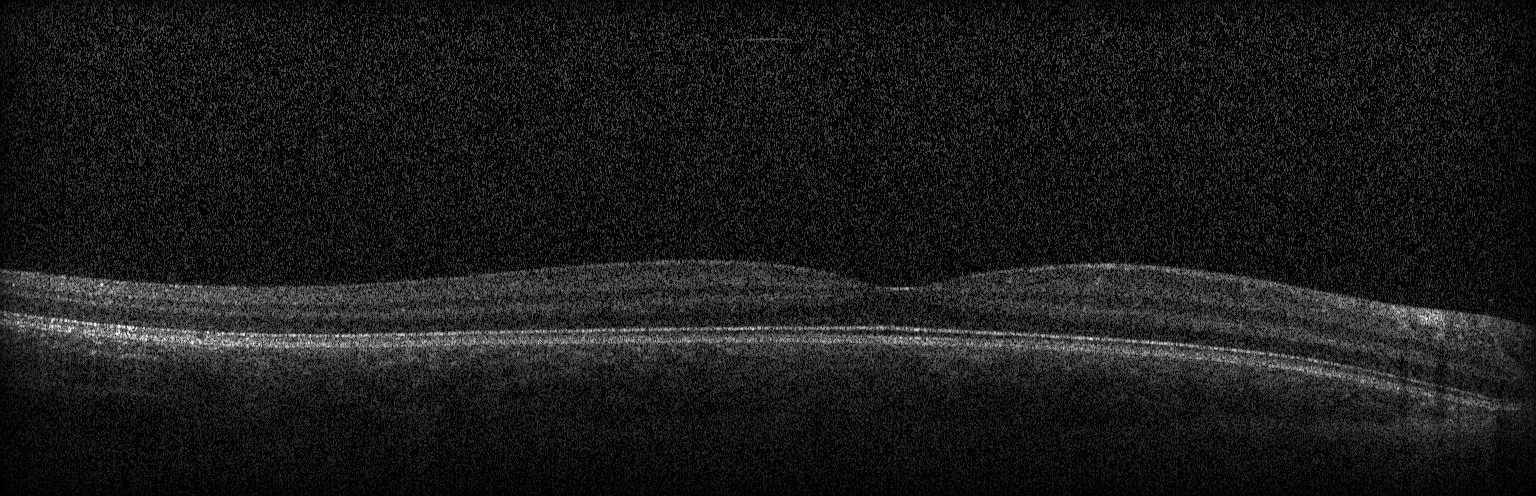
Retinal OCT cross-section. Spectral-domain optical coherence tomography. Through the macula. Acquired on a Heidelberg Spectralis — Diagnosis: no evidence of CNV, DME, or drusen.